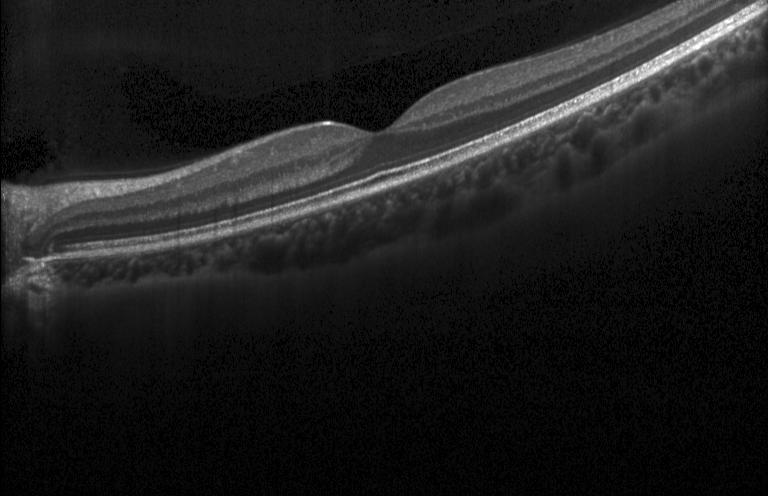

OCT finding: neither CNV, DME, nor drusen.